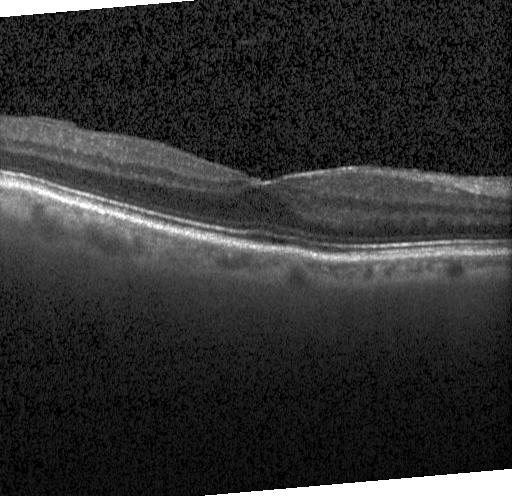 OCT scan showing no evidence of CNV, DME, or drusen.